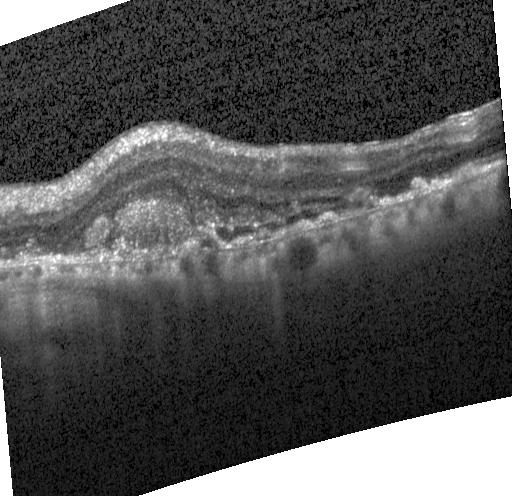 Spectral-domain optical coherence tomography; Heidelberg Spectralis; optical coherence tomography B-scan; horizontal scan through the fovea.
OCT finding: CNV.